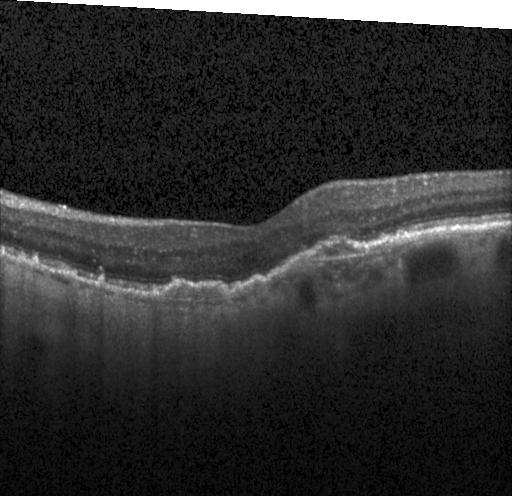

OCT B-scan. Diagnosis: choroidal neovascularization (CNV).